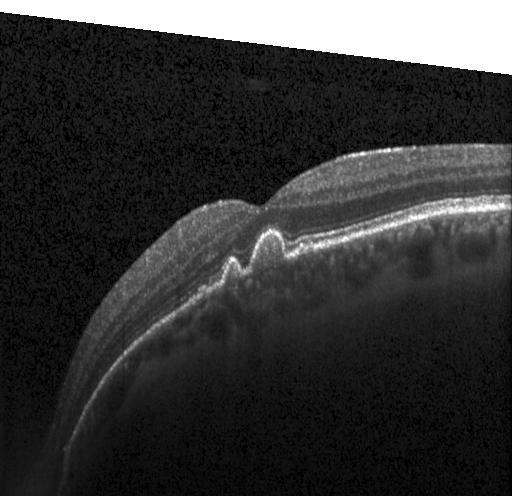

Spectral-domain optical coherence tomography · instrument: Heidelberg Spectralis · OCT B-scan — Multiple drusen.